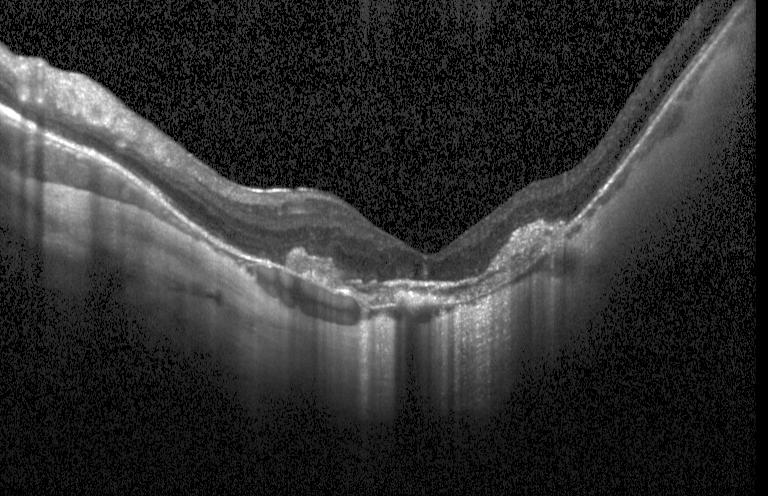

OCT line scan. Spectral-domain optical coherence tomography. Macular OCT: a choroidal neovascular membrane.